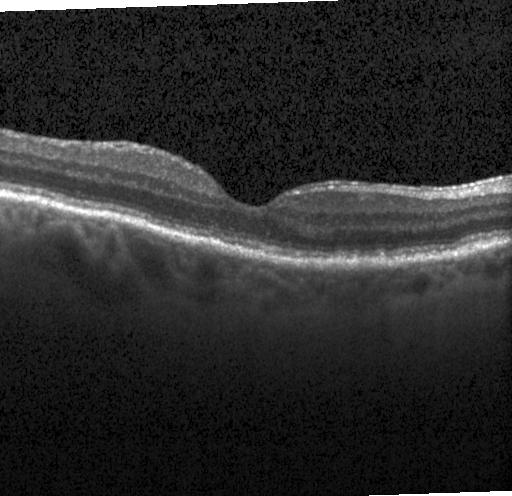

Macular OCT: neither choroidal neovascularization, diabetic macular edema, nor drusen.